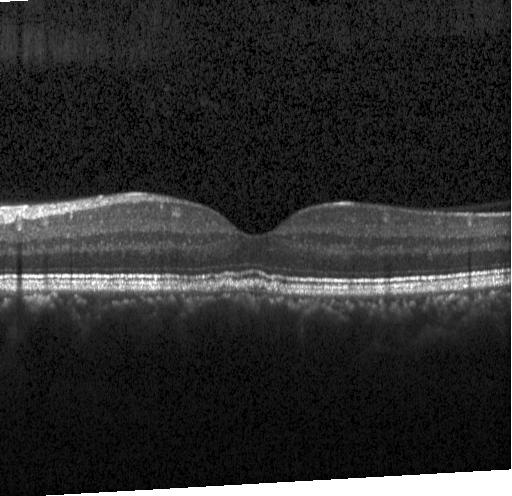
Retinal OCT cross-section.
Dx: drusen.